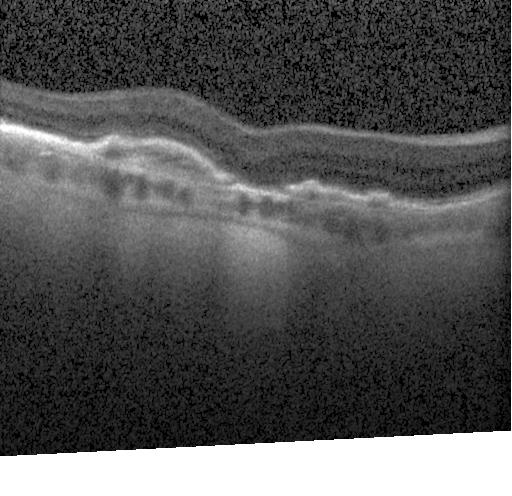

Spectral-domain OCT, instrument: Heidelberg Spectralis, optical coherence tomography B-scan
Diagnosis: choroidal neovascularization.